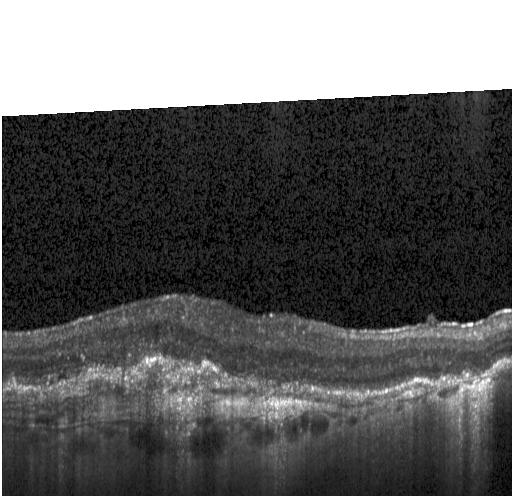

Diagnosis: a choroidal neovascular membrane.